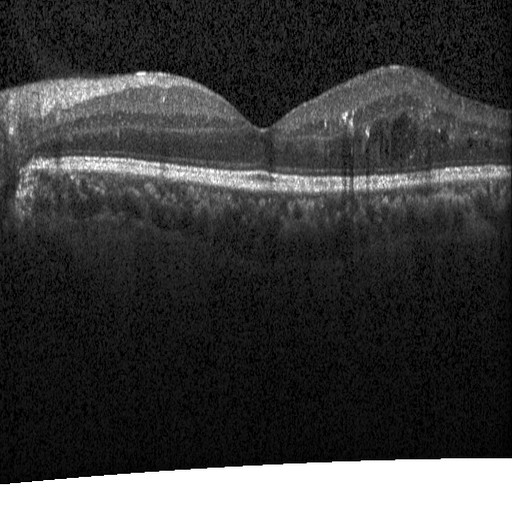

Assessment: diabetic macular edema (DME).